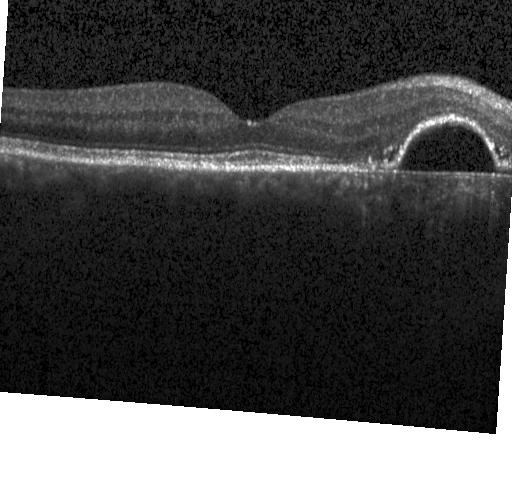
Heidelberg Spectralis OCT system · OCT B-scan · spectral-domain OCT · centered on the fovea.
Assessment: a choroidal neovascular membrane.